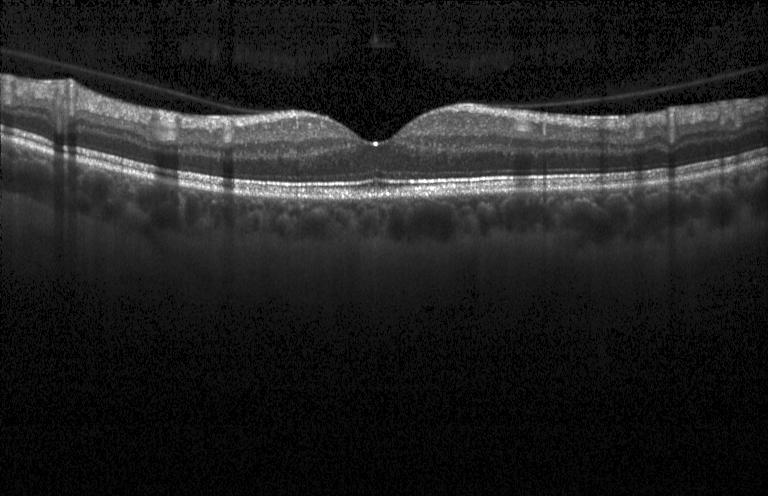
Acquired on a Heidelberg Spectralis · spectral-domain optical coherence tomography · retinal OCT B-scan · centered on the fovea.
Finding: no choroidal neovascularization, diabetic macular edema, or drusen.